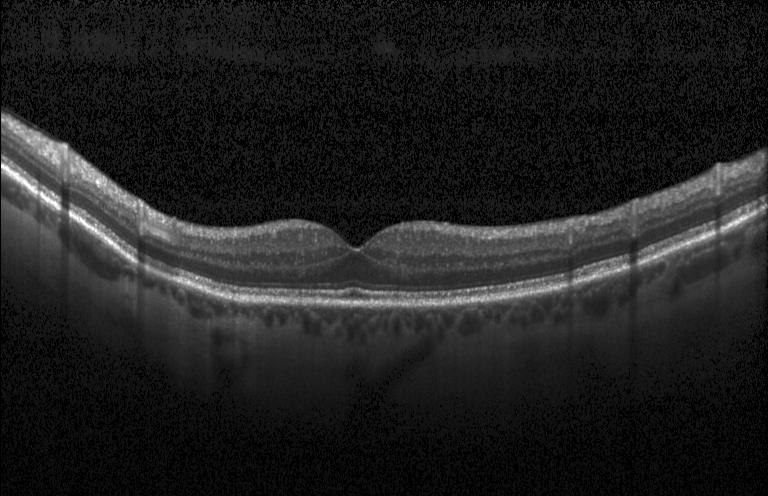

SD-OCT · OCT line scan
Dx: no evidence of CNV, DME, or drusen.